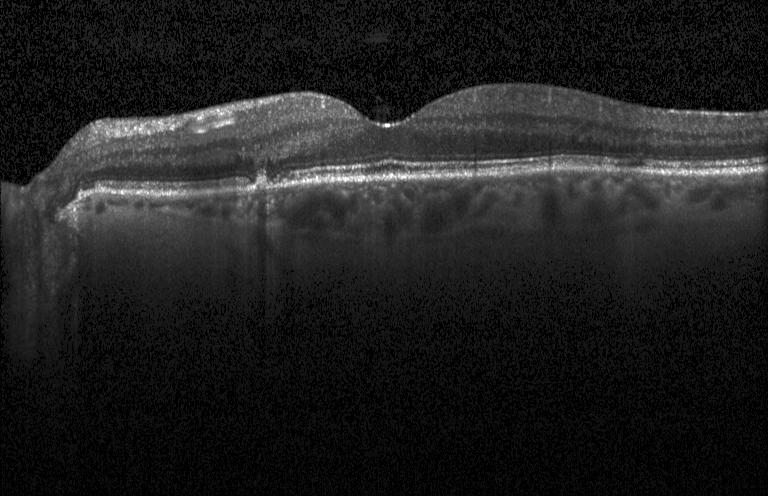
OCT B-scan, through the macula — Diagnosis: drusen.